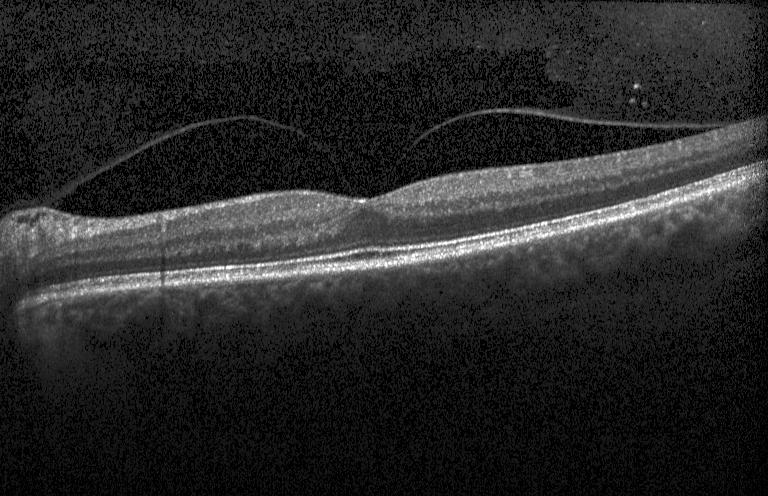

Finding: neither CNV, DME, nor drusen.